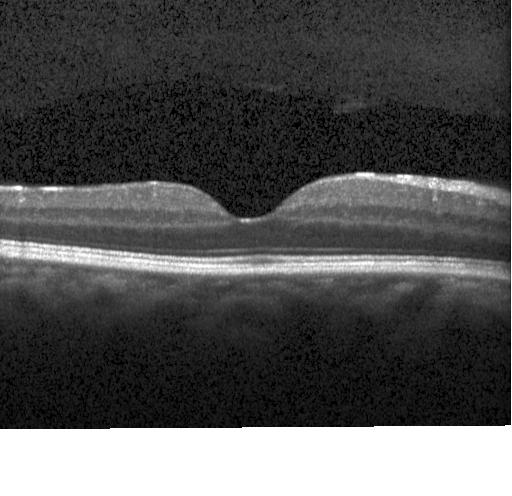
Through the macula. Instrument: Heidelberg Spectralis. Optical coherence tomography B-scan
Finding: no CNV, no DME, and no drusen.